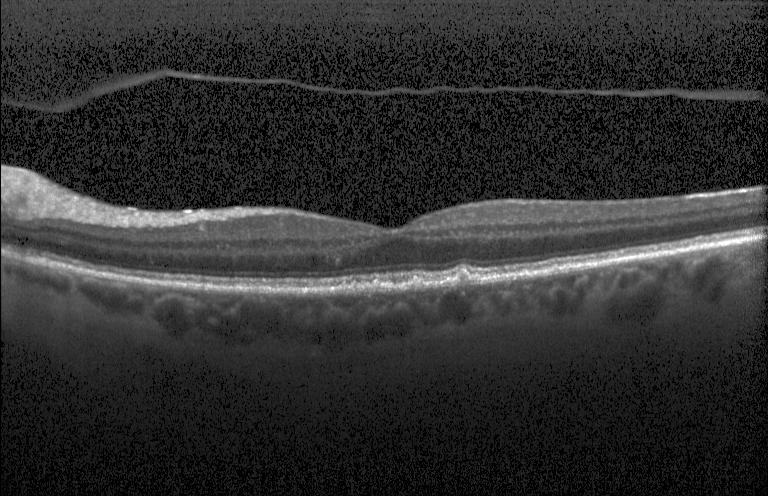

Macular scan; spectral-domain OCT; Heidelberg Spectralis OCT system; OCT B-scan.
The scan shows sub-RPE drusenoid deposits.